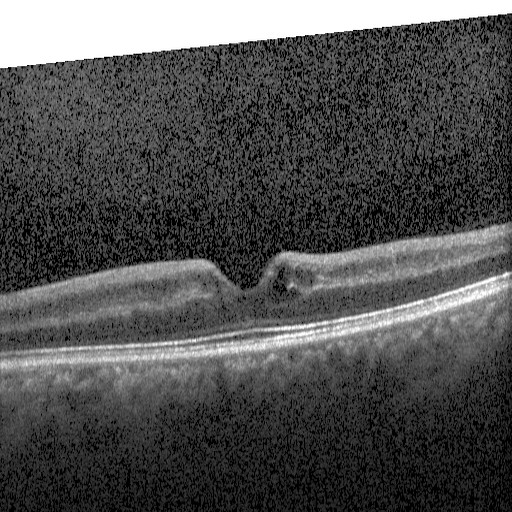 OCT finding: diabetic macular edema (DME).